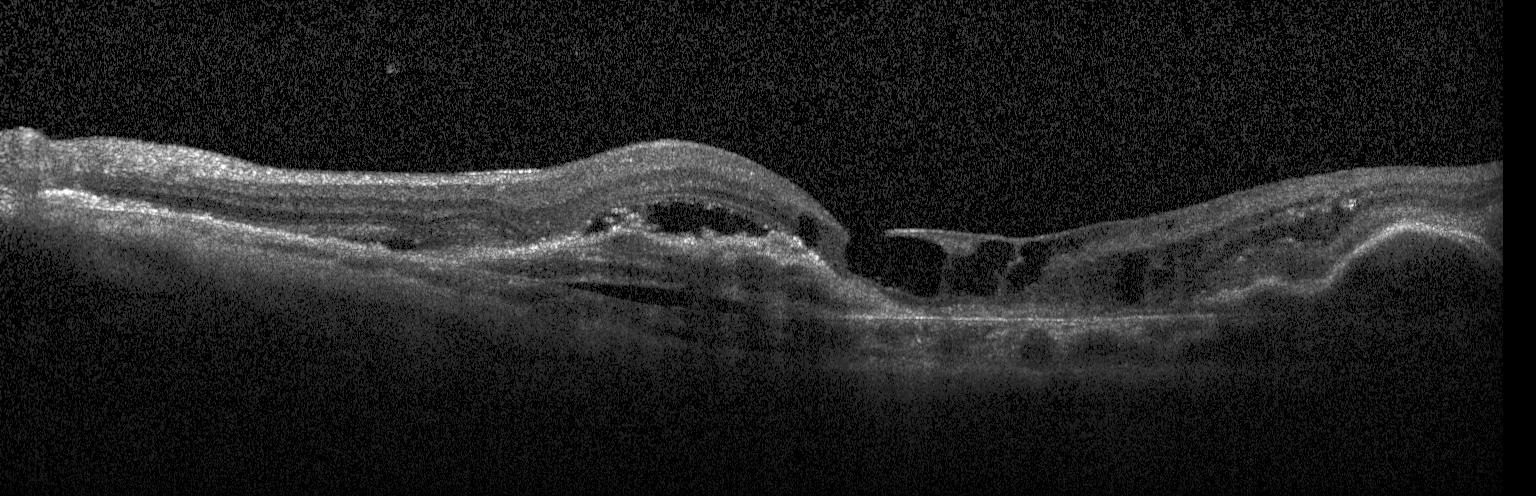
OCT B-scan showing choroidal neovascularization (CNV).